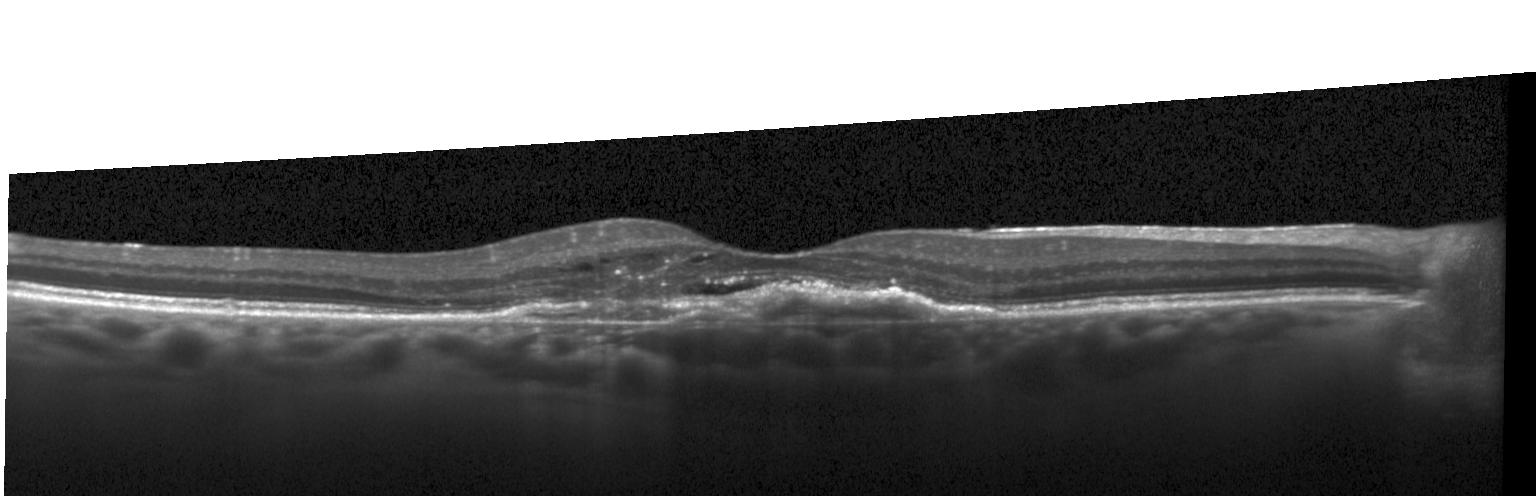

Spectral-domain OCT B-scan: a choroidal neovascular membrane.